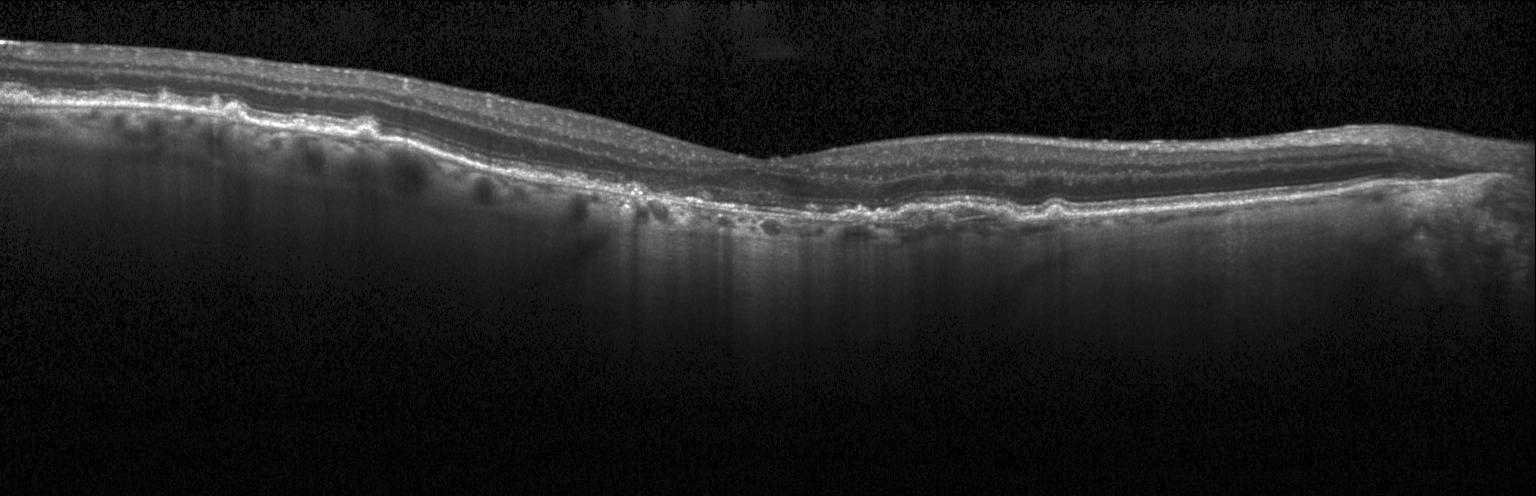
Finding: CNV.